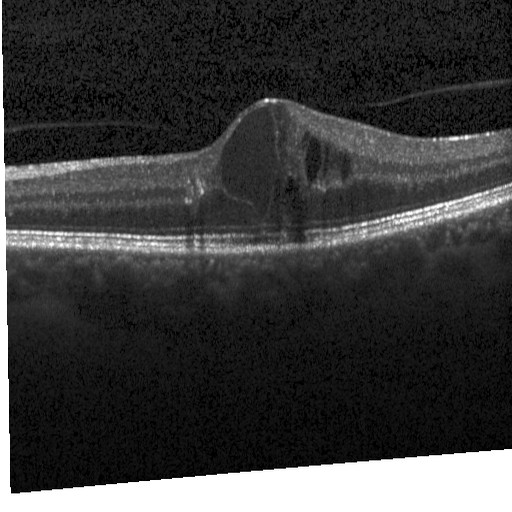 Diagnosis: DME.